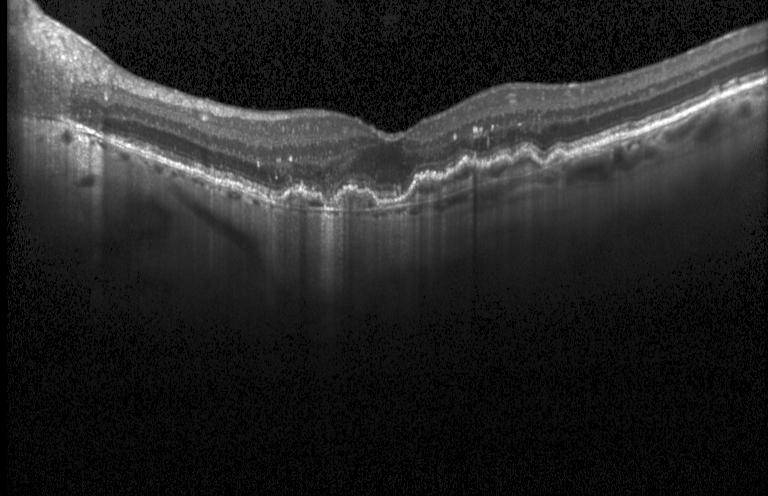
OCT scan showing choroidal neovascularization (CNV).